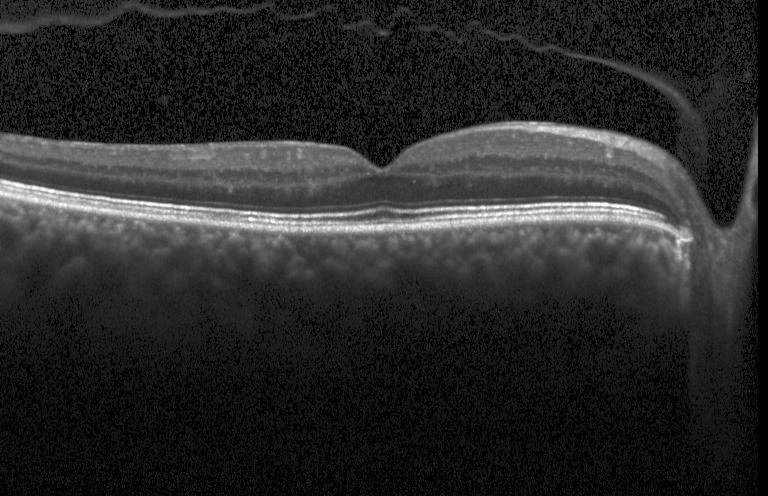
Diagnosis: neither choroidal neovascularization, diabetic macular edema, nor drusen.